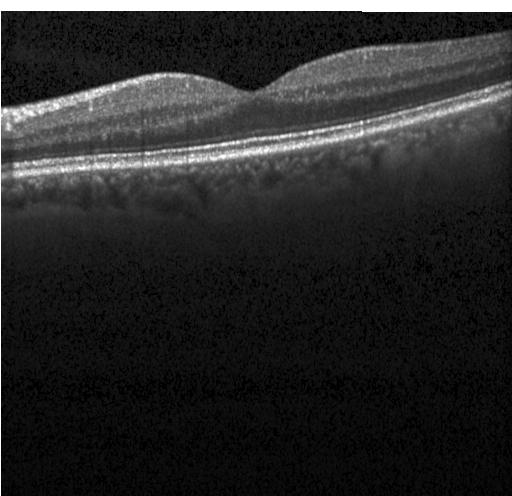 The scan shows no CNV, DME, or drusen.